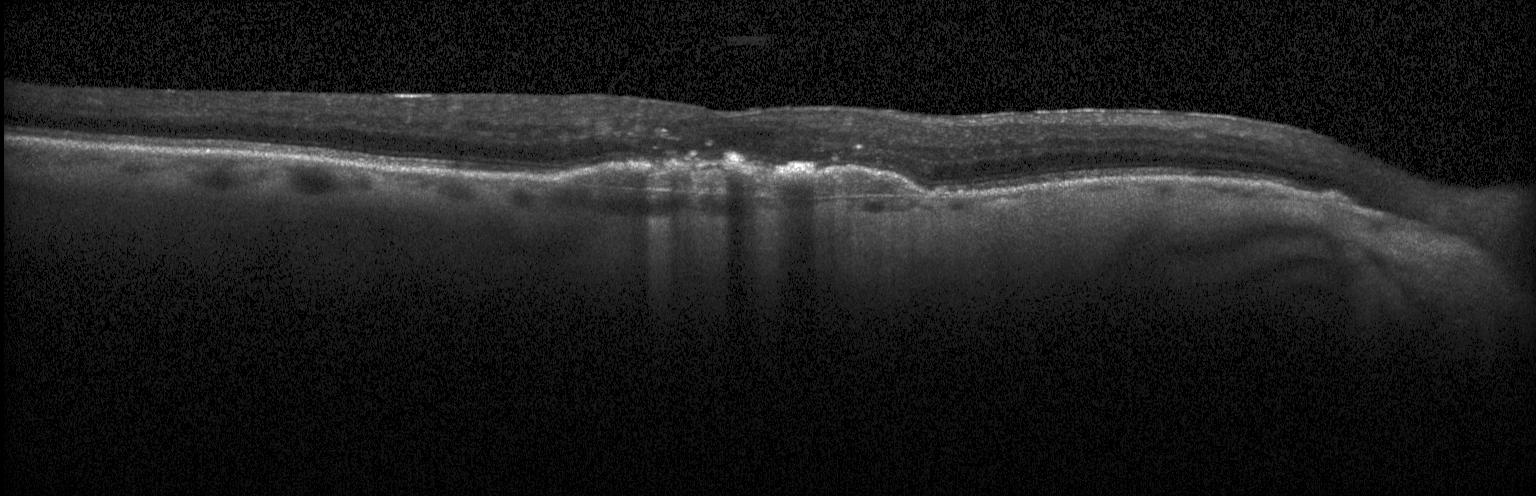

Heidelberg Spectralis OCT system, centered on the fovea, retinal OCT cross-section — Finding: a choroidal neovascular membrane.